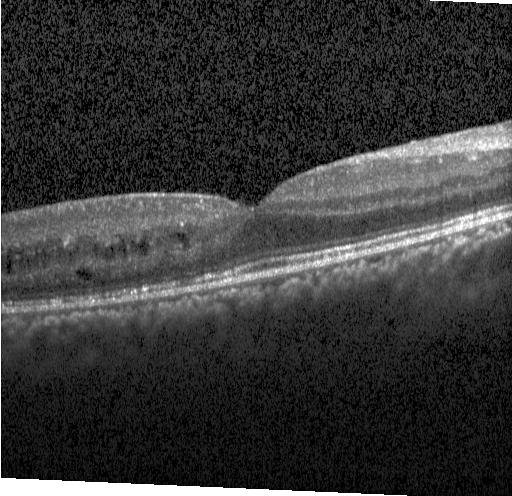 OCT B-scan showing diabetic macular edema (DME).